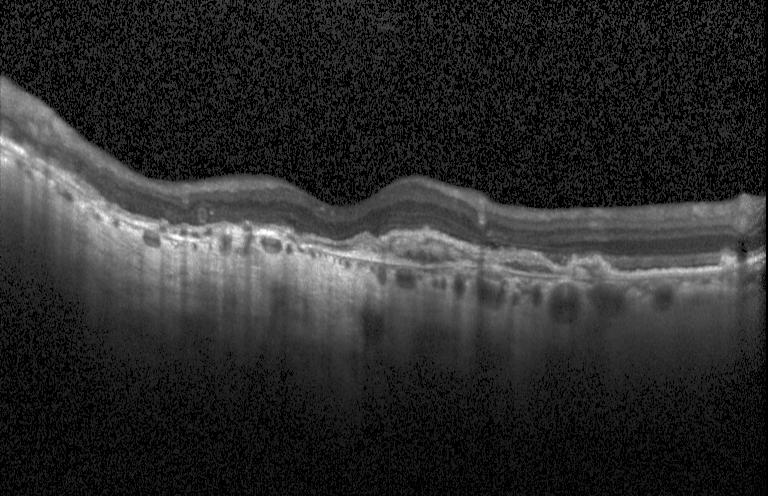

Through the macula · optical coherence tomography scan · SD-OCT — A choroidal neovascular membrane.